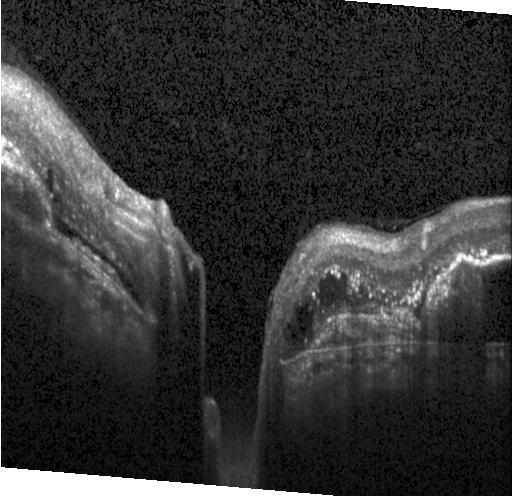

Macular scan. Optical coherence tomography B-scan. Spectral-domain optical coherence tomography — This B-scan demonstrates CNV.